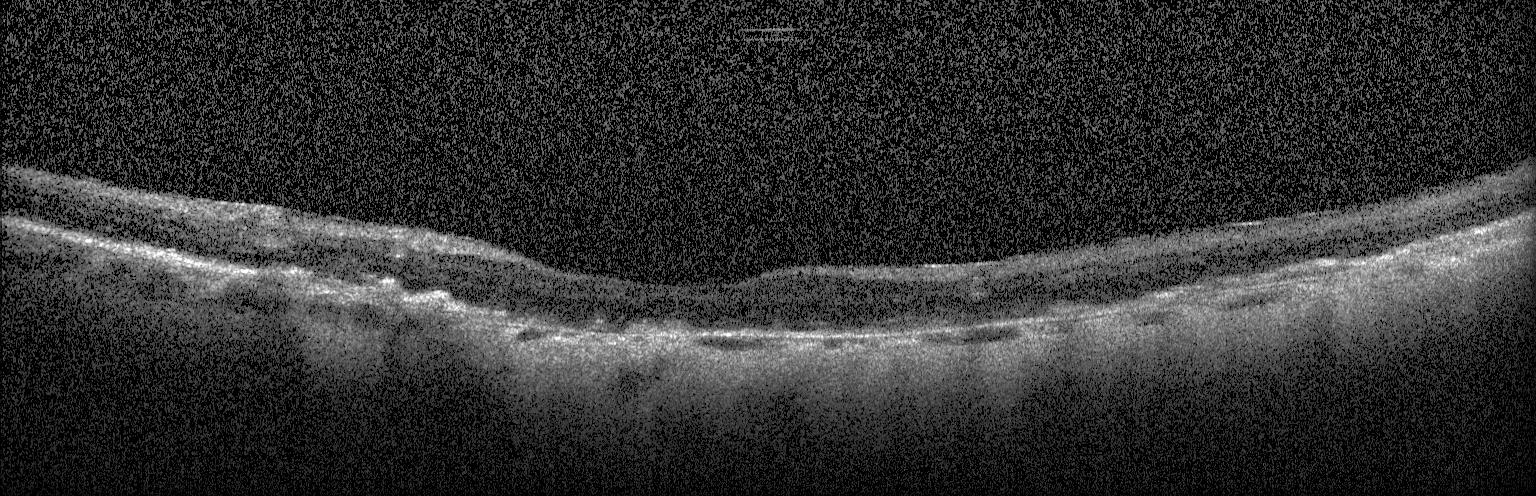
OCT line scan
OCT finding: a choroidal neovascular membrane.